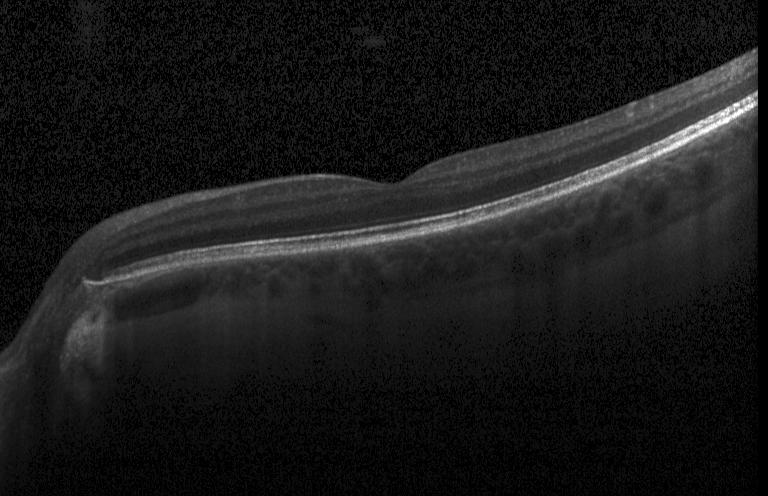 Impression: no evidence of choroidal neovascularization, diabetic macular edema, or drusen.